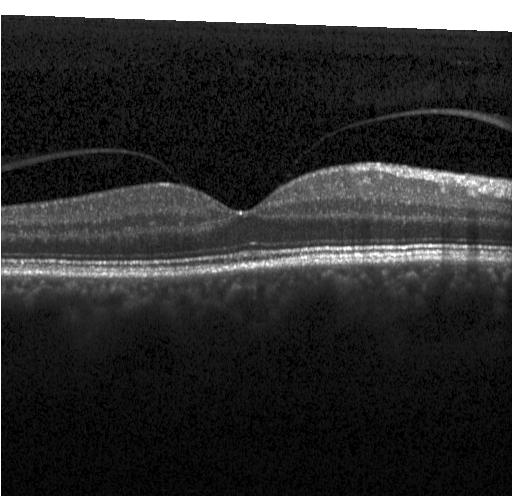
Spectral-domain OCT · retinal OCT B-scan. OCT finding: no evidence of choroidal neovascularization, diabetic macular edema, or drusen.